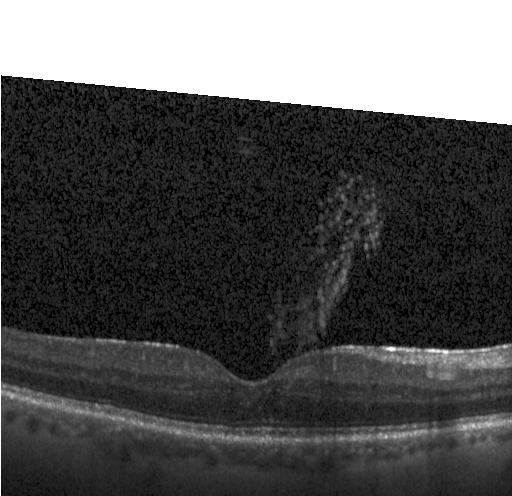
OCT line scan. Finding: no evidence of choroidal neovascularization, diabetic macular edema, or drusen.